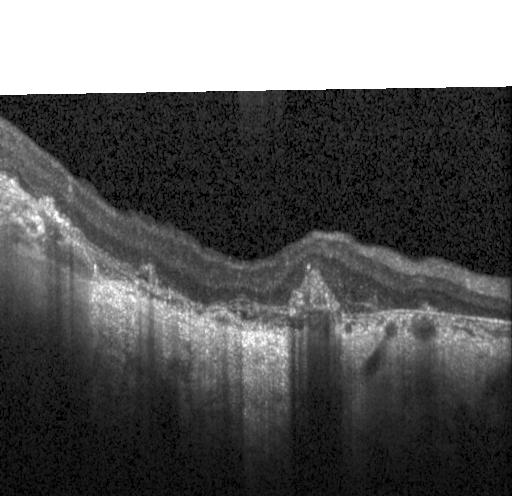
Diagnosis: CNV.